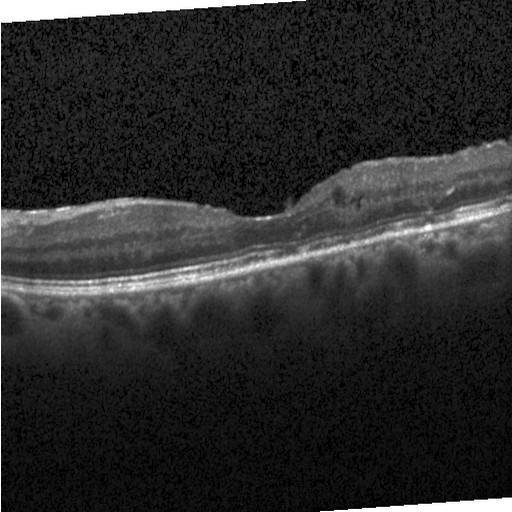
Impression: diabetic macular edema.